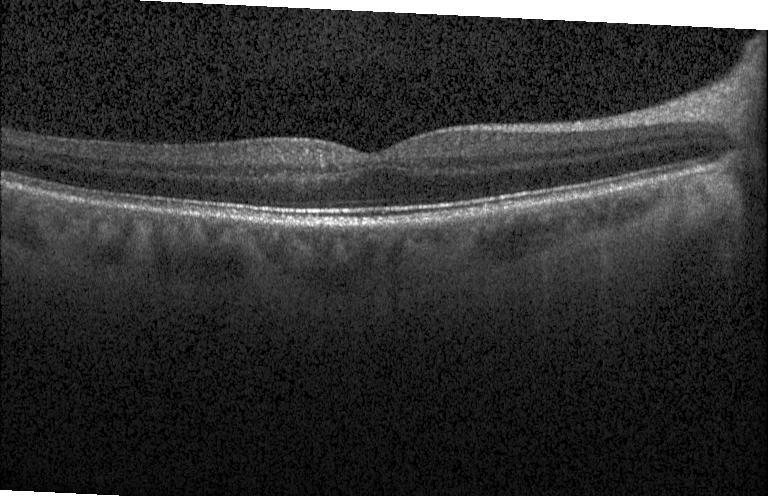 Spectral-domain optical coherence tomography · fovea-centered · acquired on a Heidelberg Spectralis · retinal OCT cross-section. The scan shows neither choroidal neovascularization, diabetic macular edema, nor drusen.